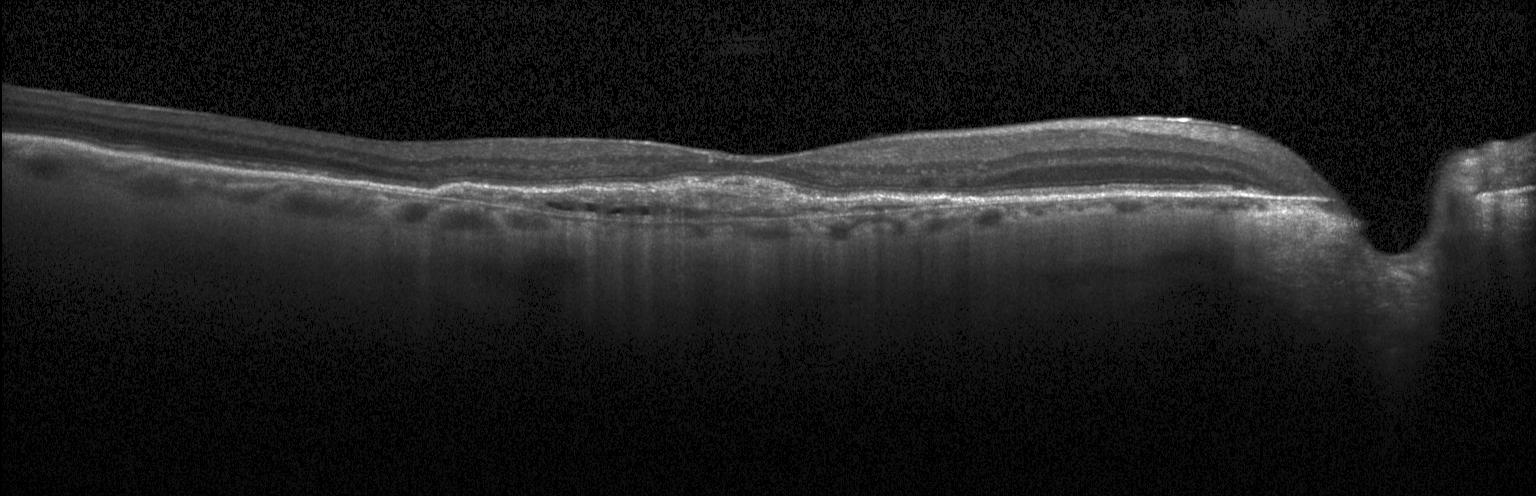

Heidelberg Spectralis, optical coherence tomography B-scan, SD-OCT. A choroidal neovascular membrane.